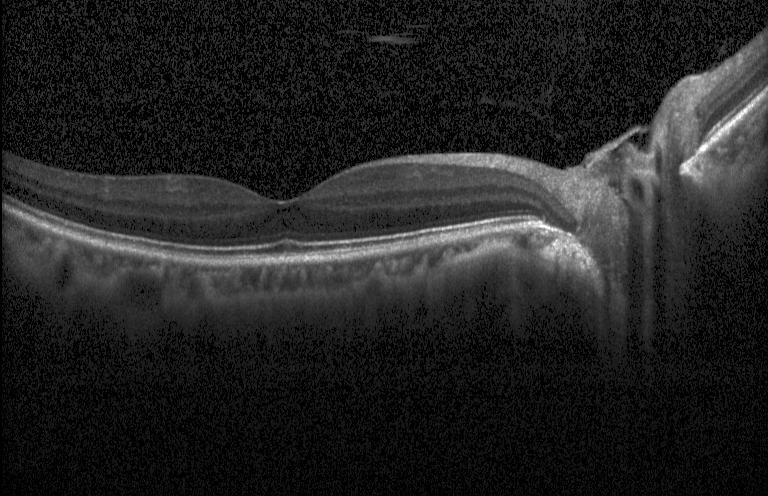 Optical coherence tomography scan; through the macula — OCT finding: no evidence of CNV, DME, or drusen.